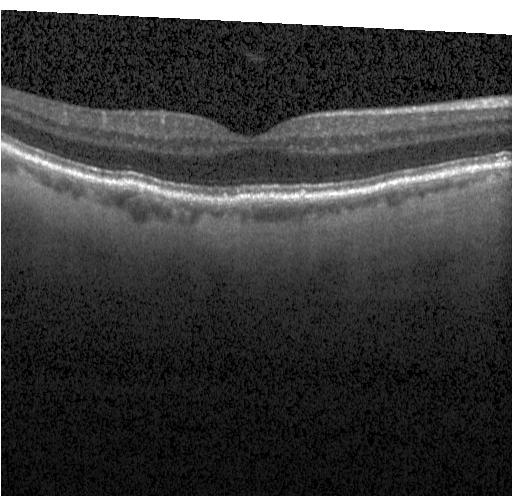 Finding: no CNV, no DME, and no drusen.